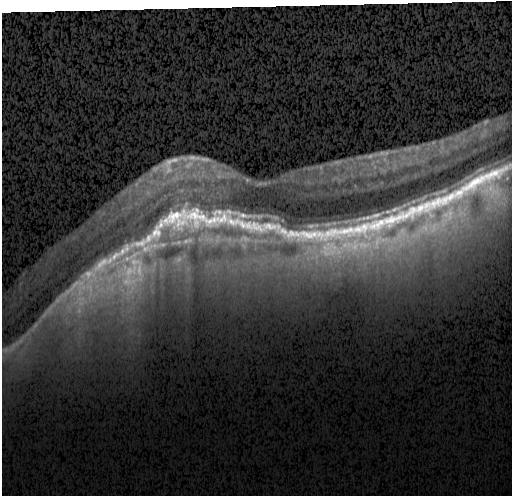 OCT scan showing a choroidal neovascular membrane.